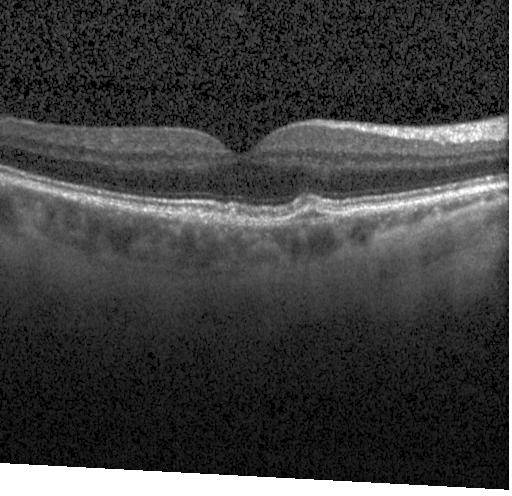 OCT B-scan.
This B-scan demonstrates sub-RPE drusenoid deposits.